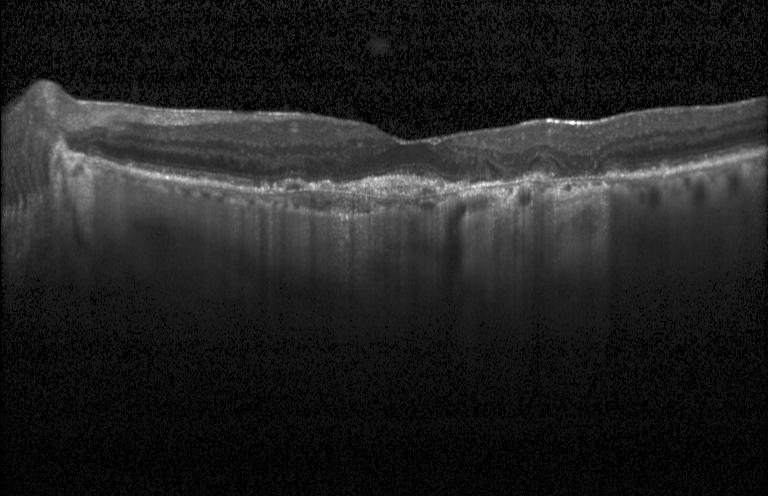
OCT line scan · acquired on a Heidelberg Spectralis
Assessment: a choroidal neovascular membrane.